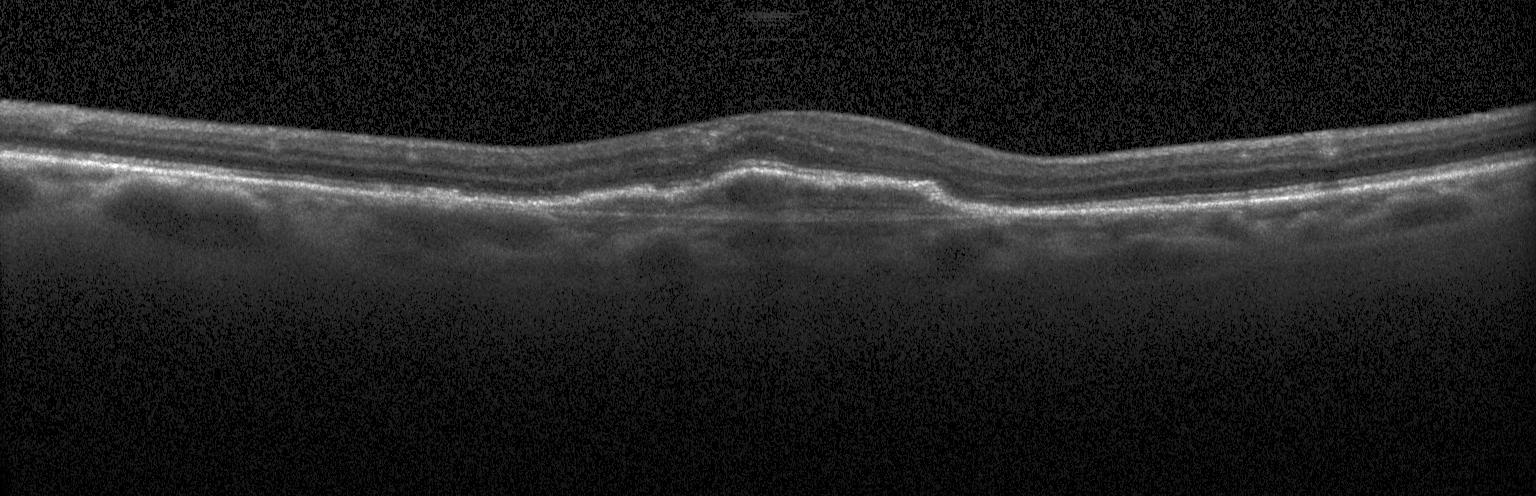 Retinal OCT B-scan; centered on the fovea — Impression: a choroidal neovascular membrane.